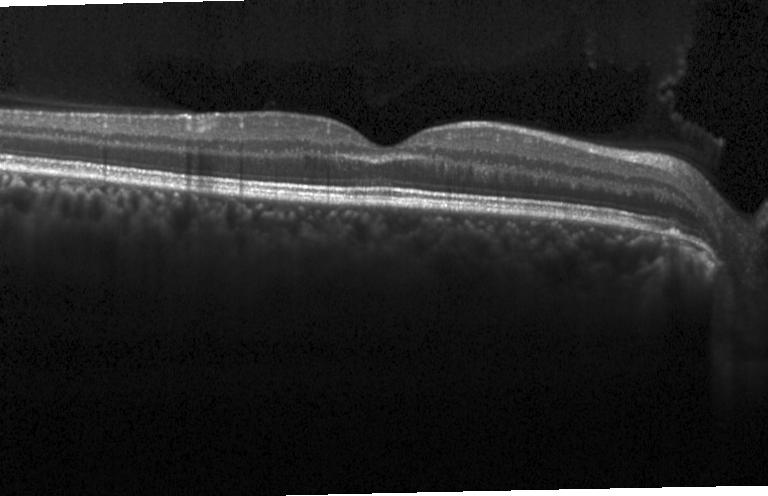

Retinal OCT cross-section; spectral-domain optical coherence tomography — Impression: no evidence of CNV, DME, or drusen.